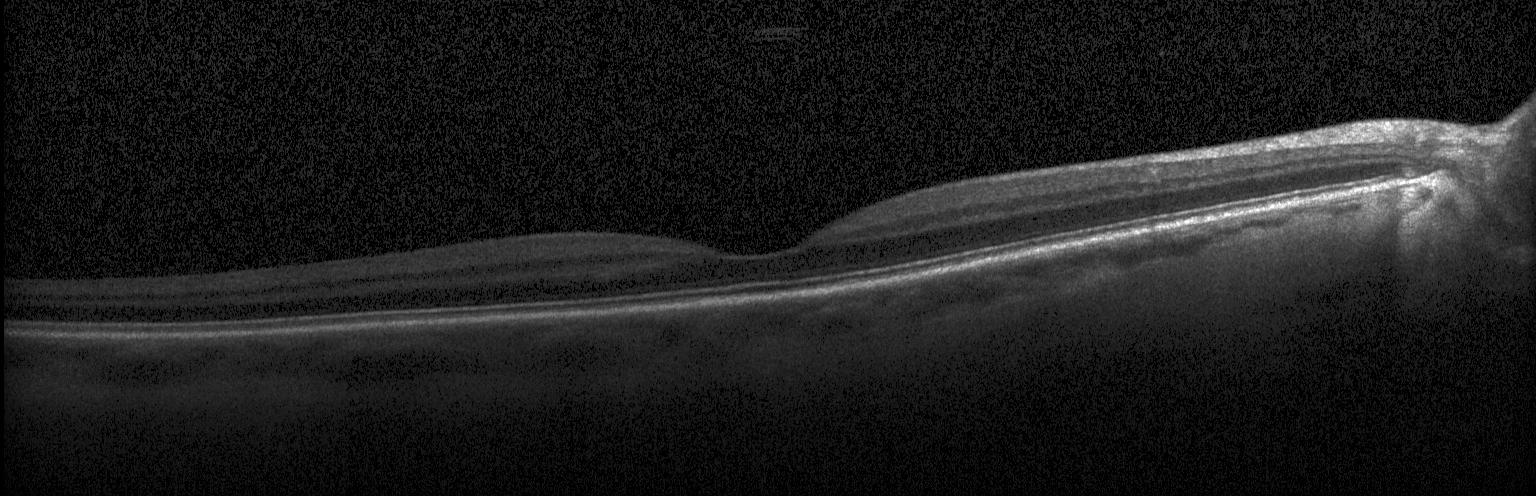

The scan shows no choroidal neovascularization, diabetic macular edema, or drusen.